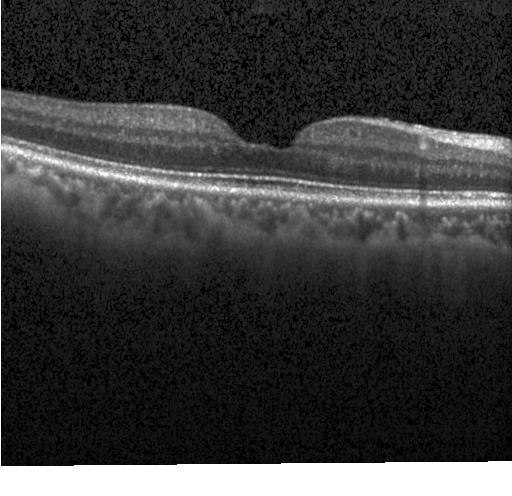
The scan shows no evidence of CNV, DME, or drusen.